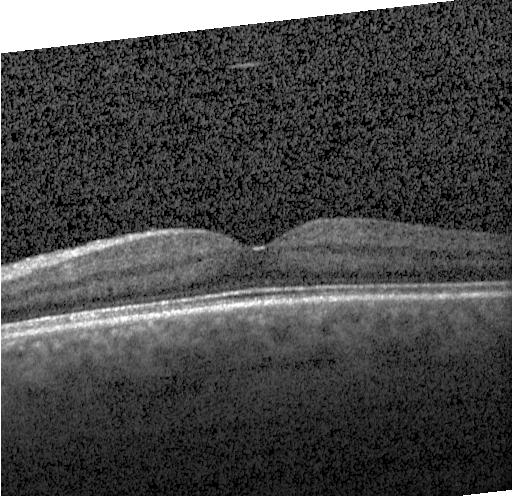

Spectral-domain OCT B-scan: no CNV, no DME, and no drusen.